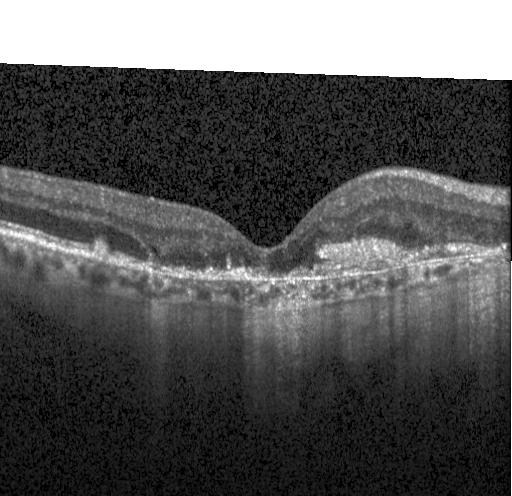 Retinal OCT B-scan — This B-scan demonstrates choroidal neovascularization.